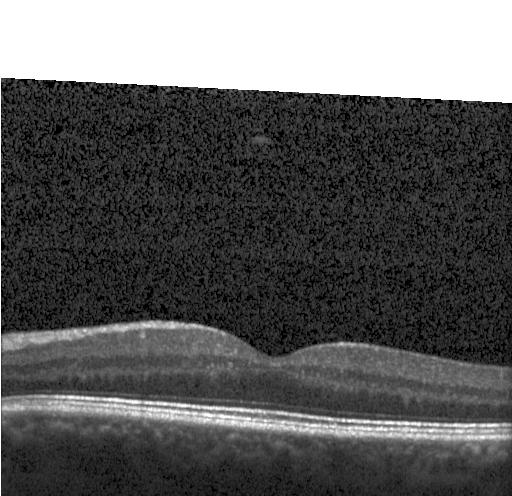
Retinal OCT cross-section; acquired on a Heidelberg Spectralis
Impression: no choroidal neovascularization, no diabetic macular edema, and no drusen.